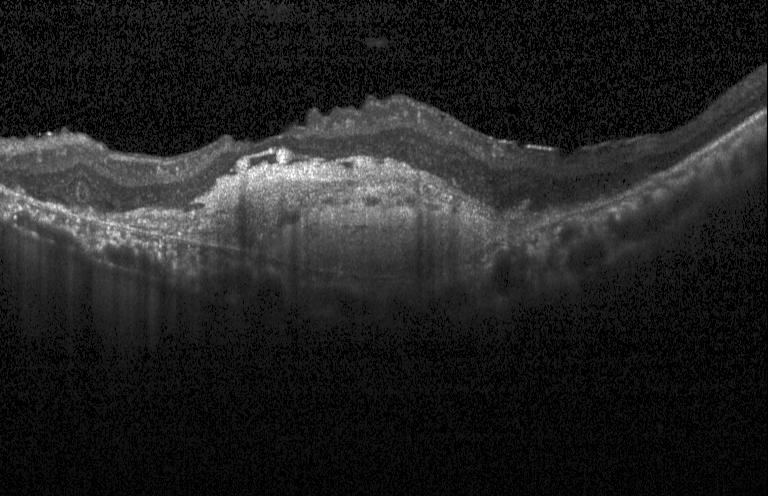 Spectral-domain optical coherence tomography, instrument: Heidelberg Spectralis, retinal OCT B-scan.
Impression: choroidal neovascularization.